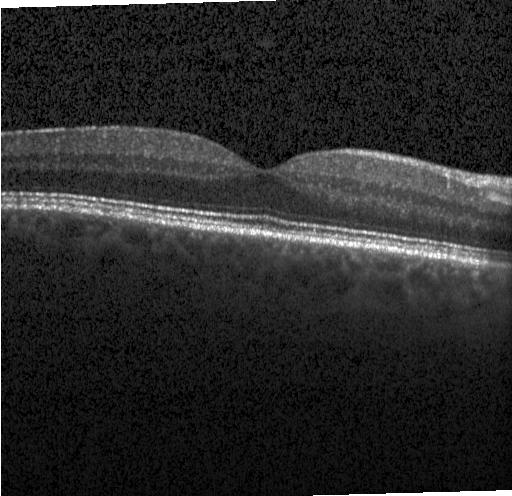

Spectral-domain OCT B-scan: no evidence of CNV, DME, or drusen.